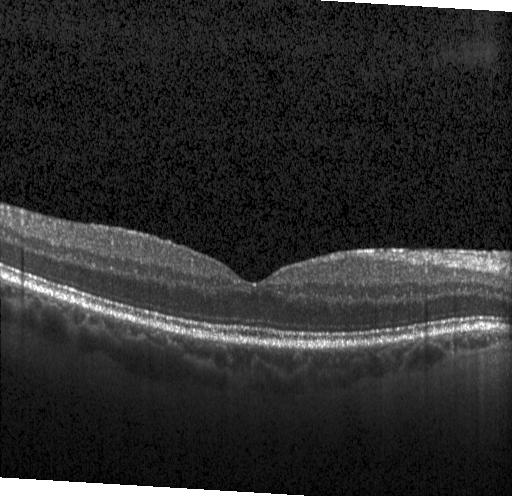 Finding: no CNV, no DME, and no drusen.